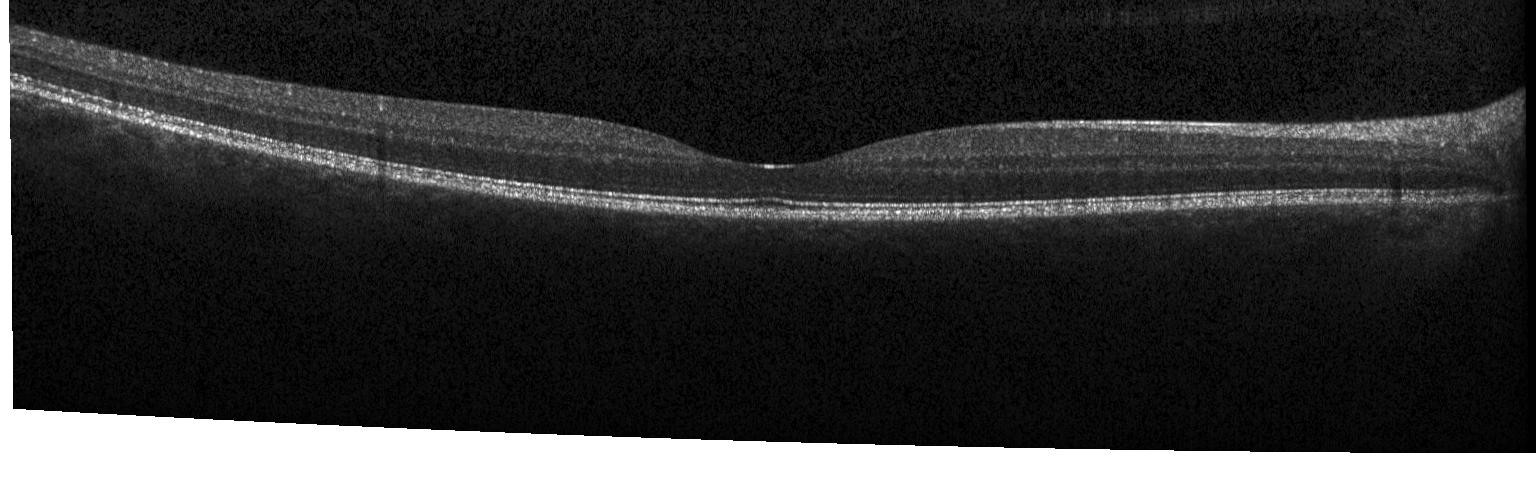

Horizontal scan through the fovea. SD-OCT. OCT line scan
Impression: no evidence of choroidal neovascularization, diabetic macular edema, or drusen.